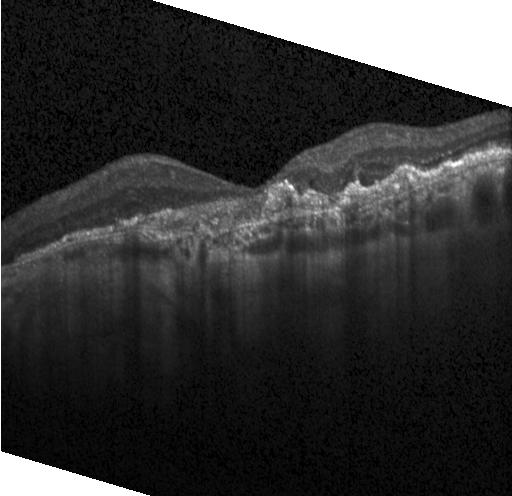 Spectral-domain OCT. Optical coherence tomography scan. Macular OCT: a choroidal neovascular membrane.